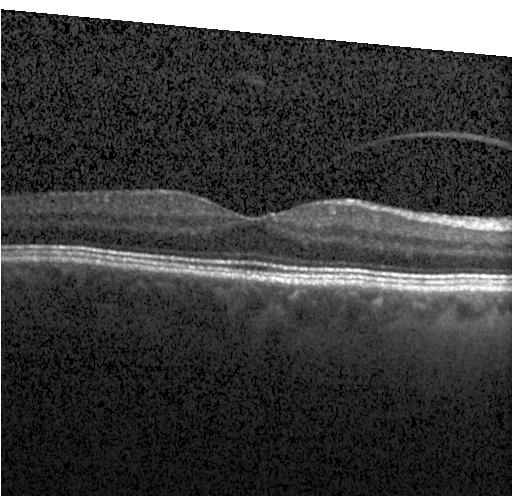
Horizontal scan through the fovea, retinal OCT B-scan, Heidelberg Spectralis, SD-OCT — Diagnosis: neither CNV, DME, nor drusen.